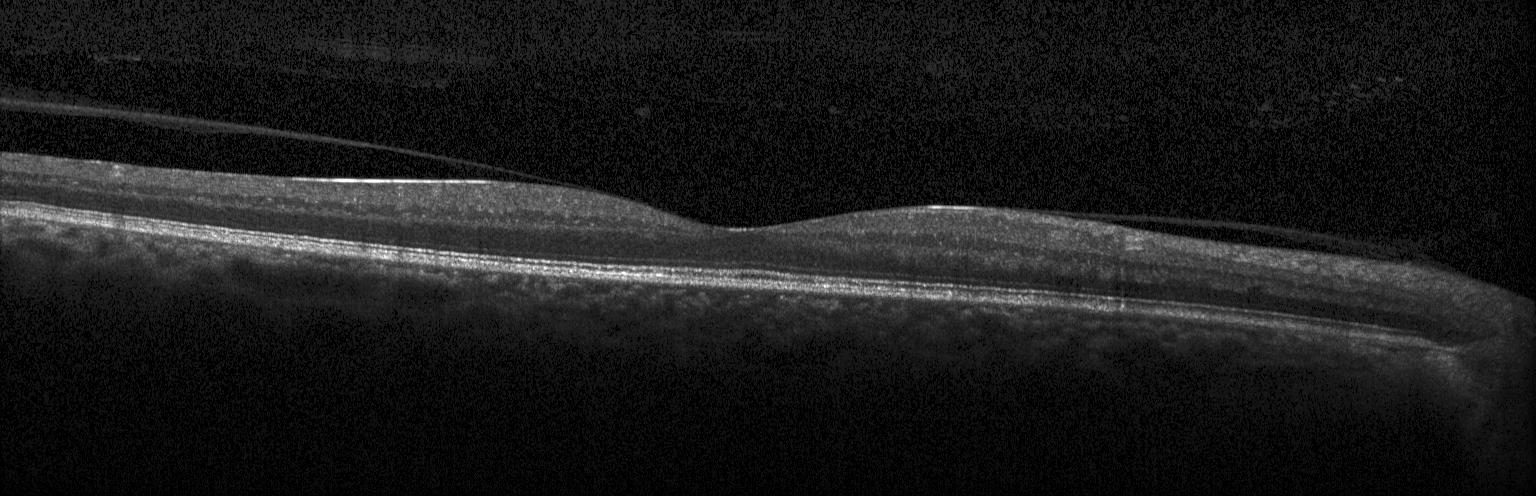
Impression: no CNV, no DME, and no drusen.